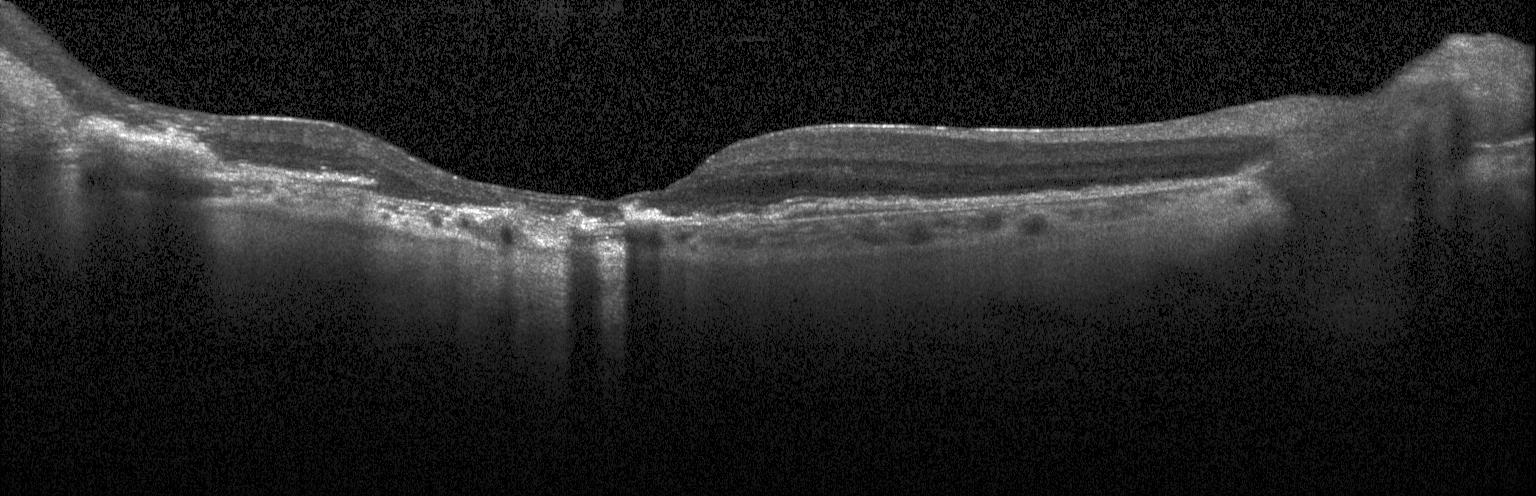
Heidelberg Spectralis; OCT line scan.
This B-scan demonstrates a choroidal neovascular membrane.